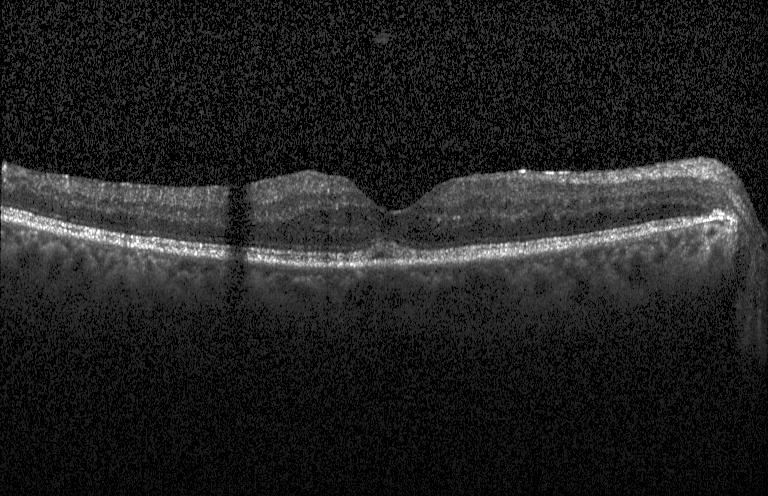
Instrument: Heidelberg Spectralis; spectral-domain OCT; macular scan; OCT line scan — Impression: diabetic macular edema (DME).